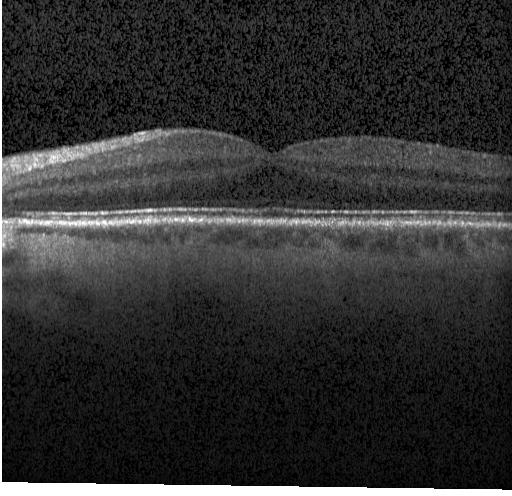

Impression: neither choroidal neovascularization, diabetic macular edema, nor drusen.